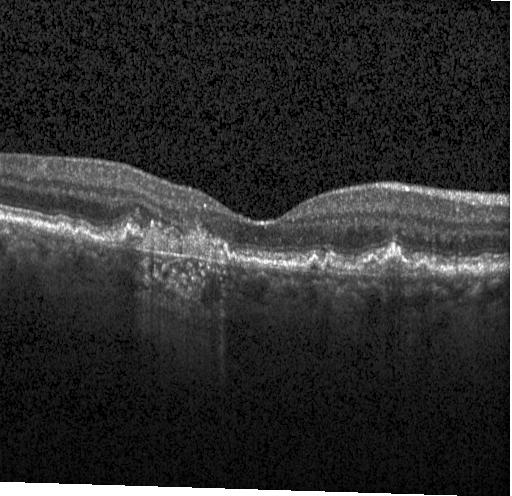
CNV.